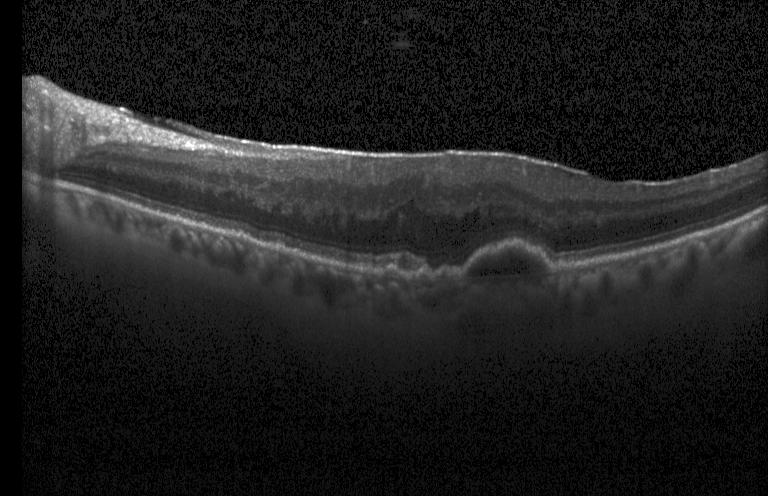 Optical coherence tomography B-scan.
Macular OCT: a choroidal neovascular membrane.